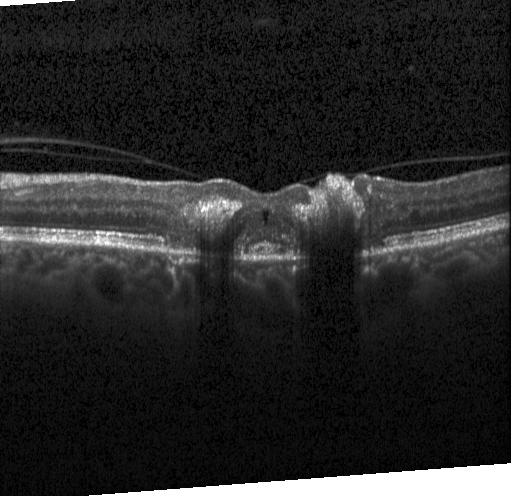
Optical coherence tomography scan. Finding: choroidal neovascularization (CNV).